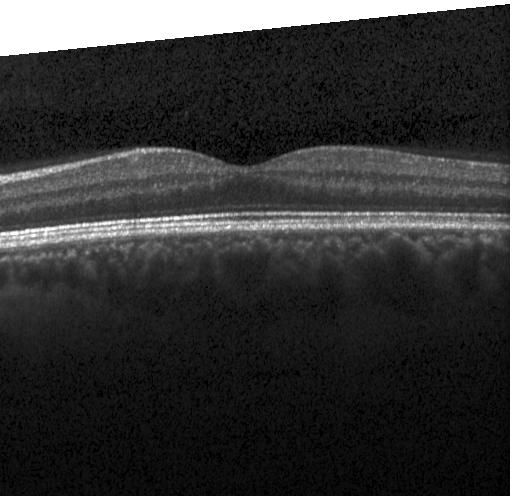
OCT B-scan.
Finding: neither choroidal neovascularization, diabetic macular edema, nor drusen.